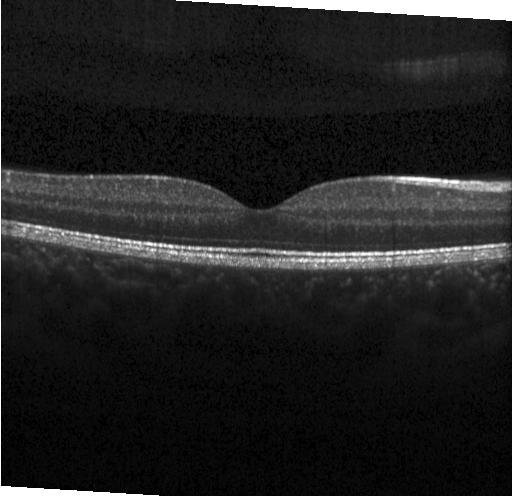 Horizontal scan through the fovea. Heidelberg Spectralis OCT system. Spectral-domain optical coherence tomography. OCT line scan. Assessment: no choroidal neovascularization, diabetic macular edema, or drusen.